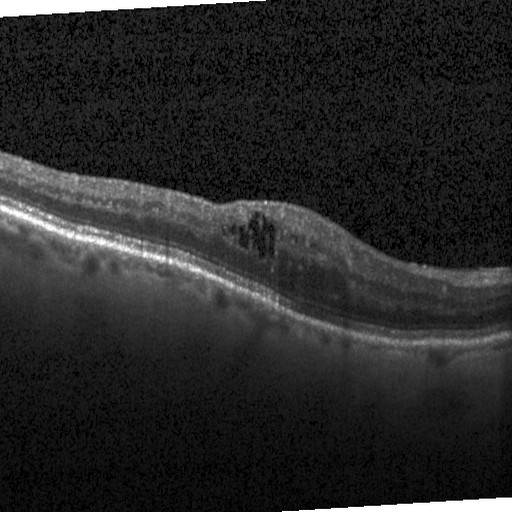

Spectral-domain OCT. Optical coherence tomography B-scan — OCT finding: diabetic macular edema (DME).